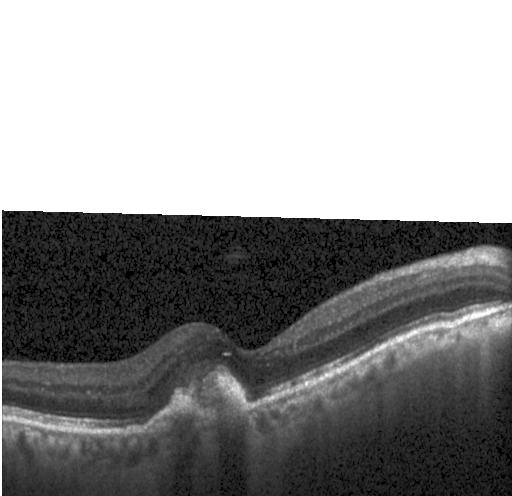

Heidelberg Spectralis, retinal OCT cross-section, fovea-centered
Finding: CNV.